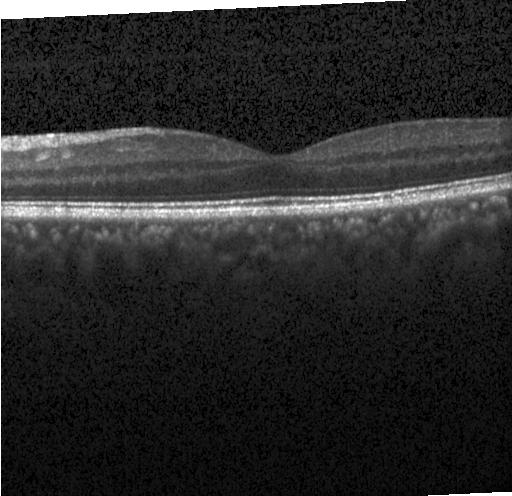 Optical coherence tomography scan
Impression: no evidence of choroidal neovascularization, diabetic macular edema, or drusen.